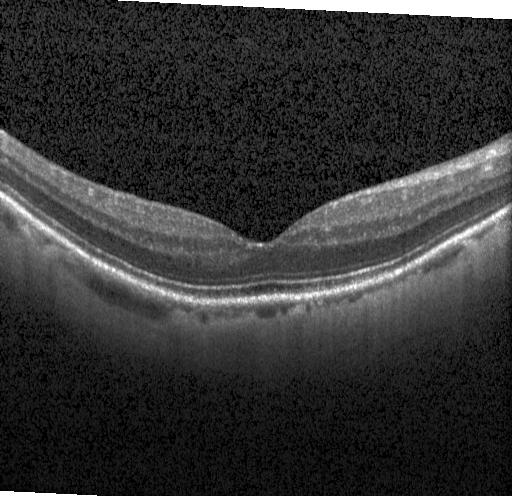
Retinal OCT cross-section.
Assessment: no evidence of choroidal neovascularization, diabetic macular edema, or drusen.